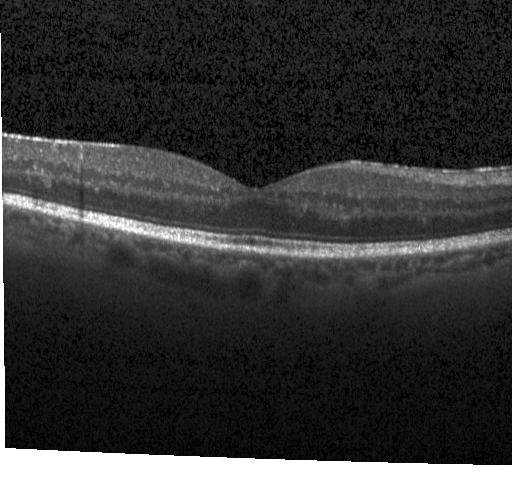

Finding: no evidence of choroidal neovascularization, diabetic macular edema, or drusen.